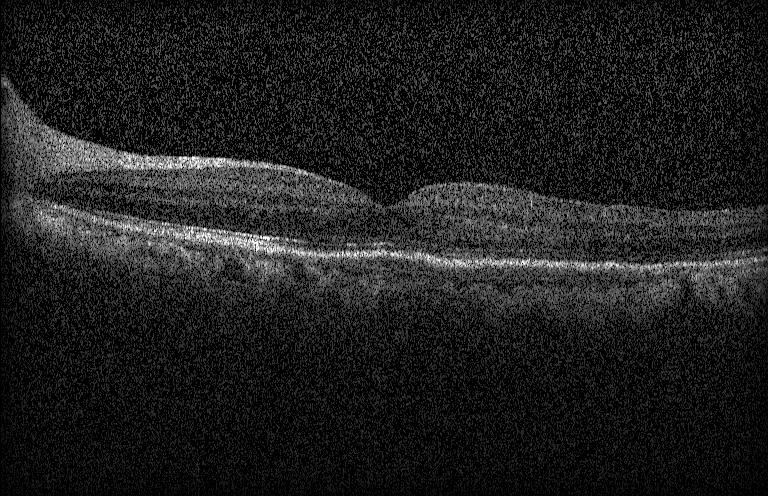 Assessment: neither choroidal neovascularization, diabetic macular edema, nor drusen.